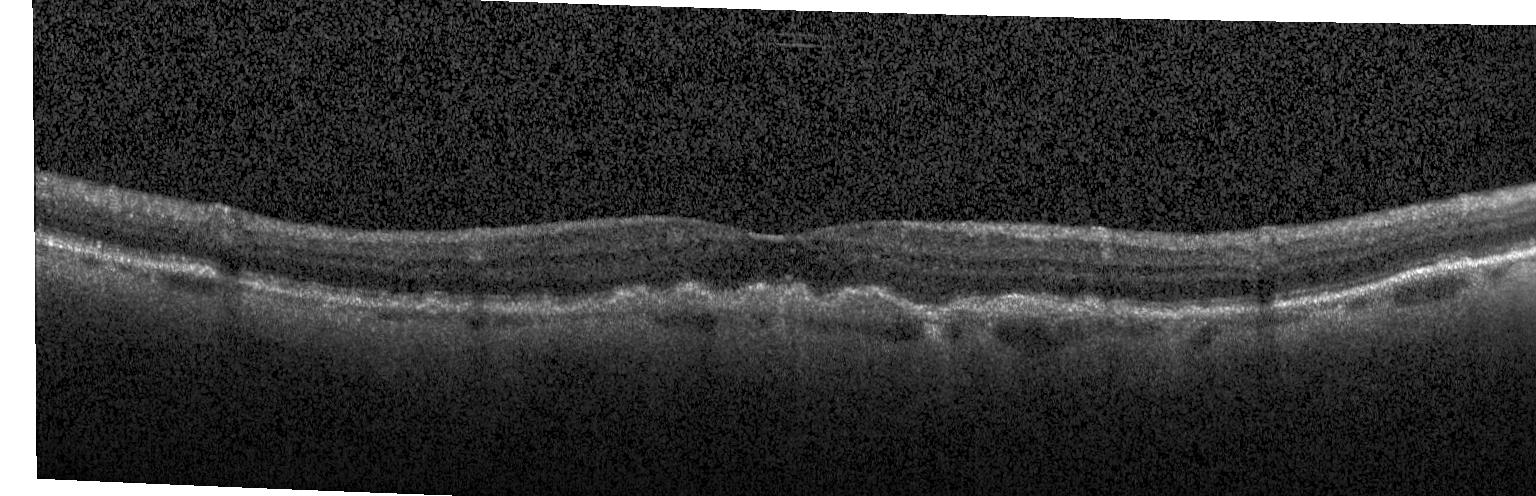 OCT finding: a choroidal neovascular membrane.